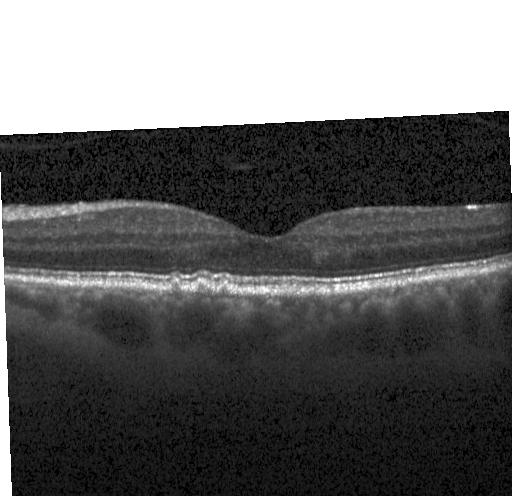 Finding: sub-RPE drusenoid deposits.